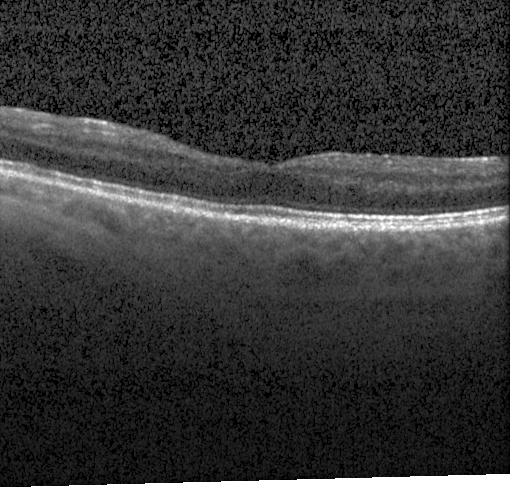 Retinal OCT B-scan — Macular OCT: no choroidal neovascularization, diabetic macular edema, or drusen.